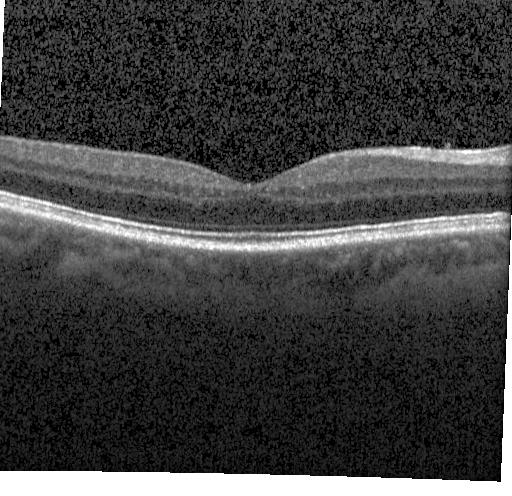
Macular scan; OCT B-scan. Assessment: neither choroidal neovascularization, diabetic macular edema, nor drusen.